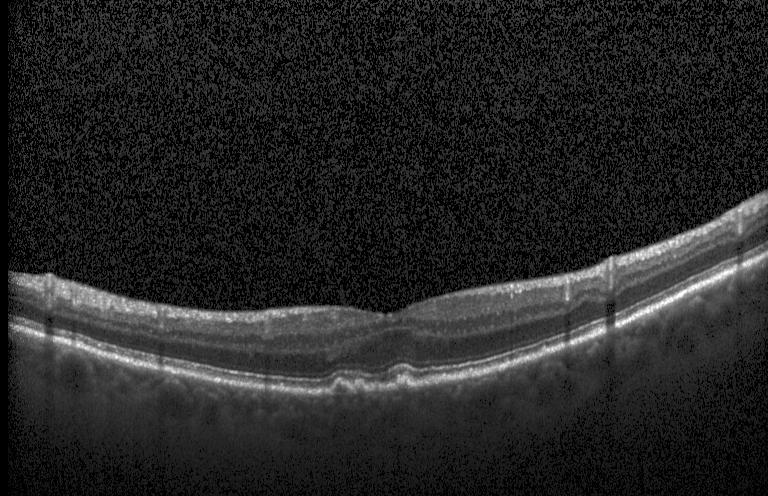
Macular OCT: drusen.